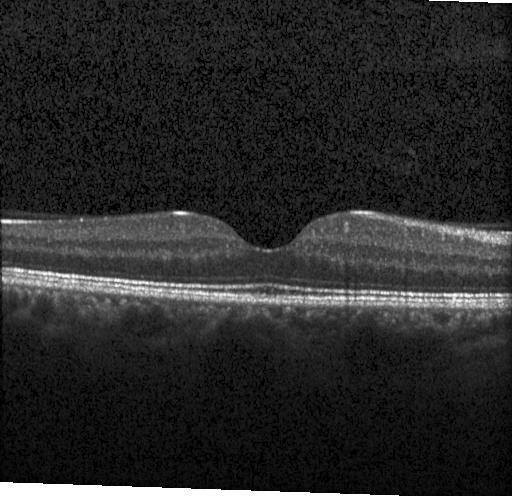 Fovea-centered, optical coherence tomography B-scan, Heidelberg Spectralis OCT system — Impression: no choroidal neovascularization, diabetic macular edema, or drusen.